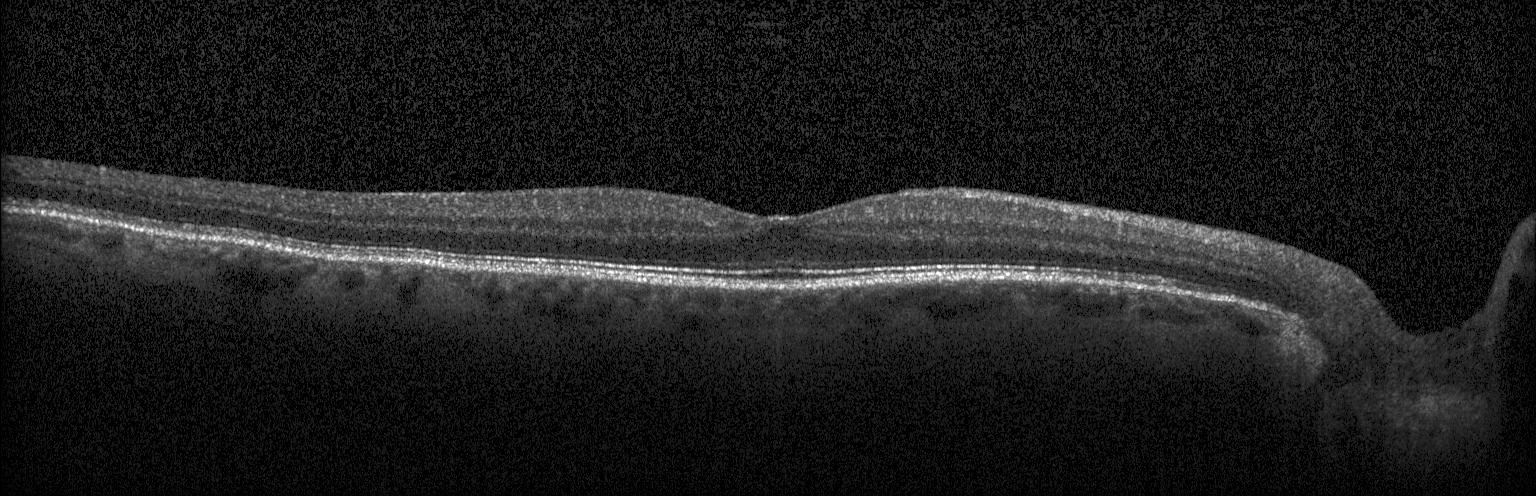
Heidelberg Spectralis; retinal OCT B-scan; spectral-domain optical coherence tomography
Impression: no evidence of CNV, DME, or drusen.